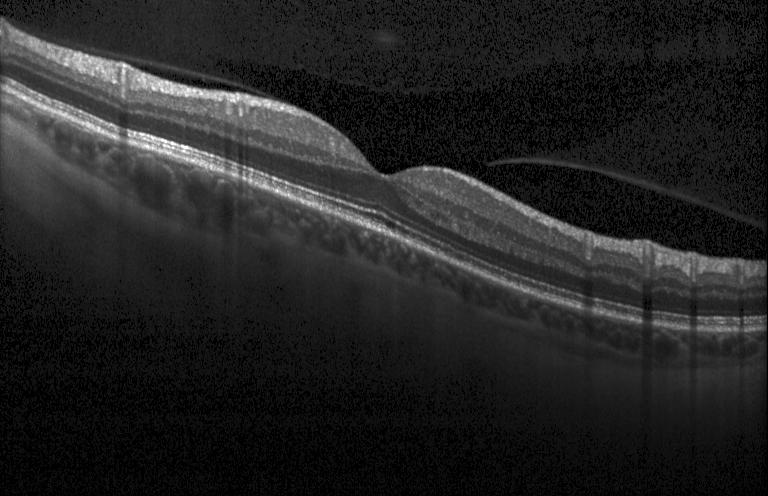
Fovea-centered, retinal OCT cross-section — No choroidal neovascularization, no diabetic macular edema, and no drusen.